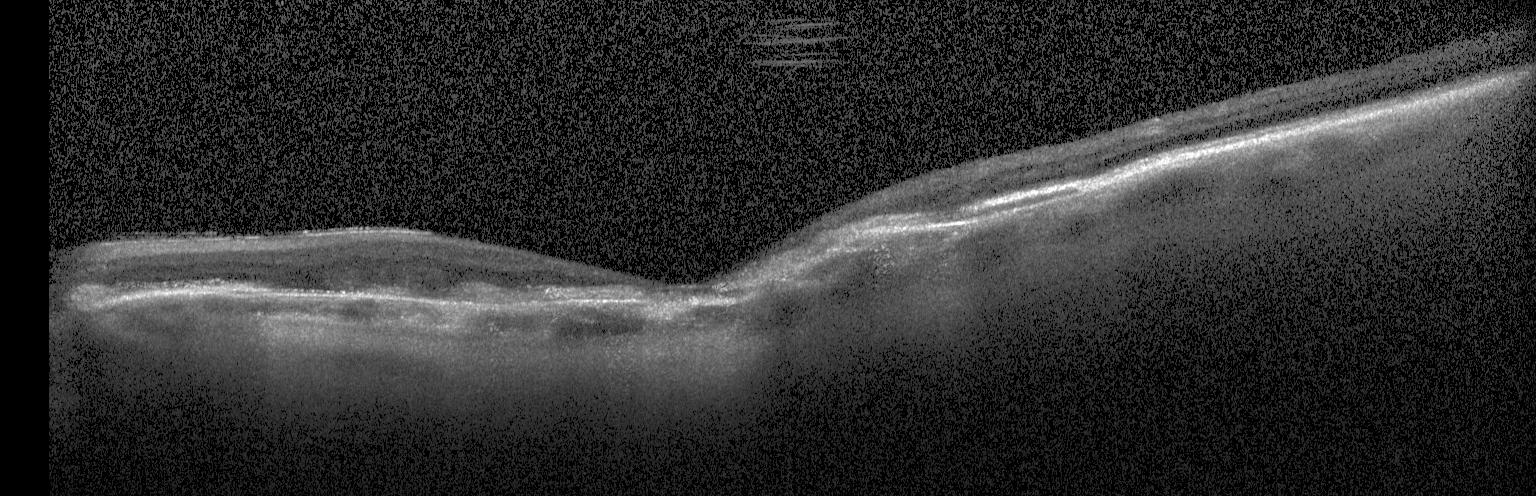
Retinal OCT cross-section — Diagnosis: a choroidal neovascular membrane.